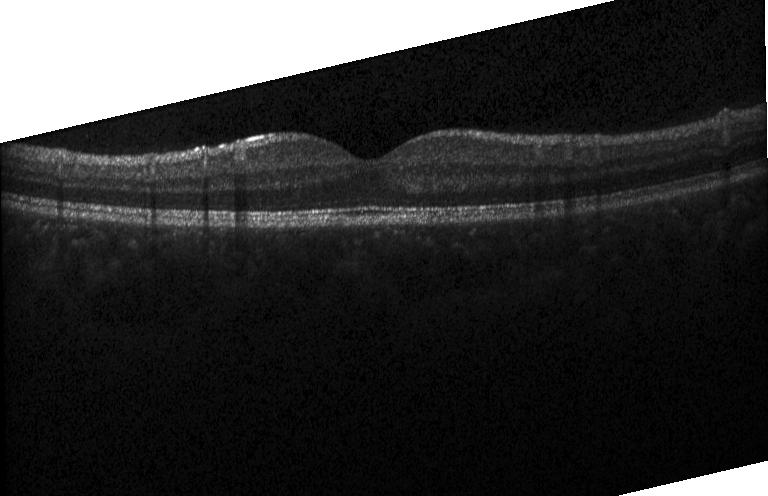
OCT B-scan.
Finding: neither CNV, DME, nor drusen.